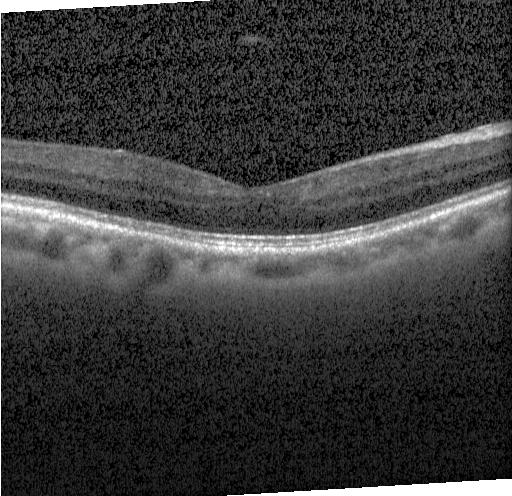

Fovea-centered · retinal OCT cross-section. OCT finding: no evidence of choroidal neovascularization, diabetic macular edema, or drusen.